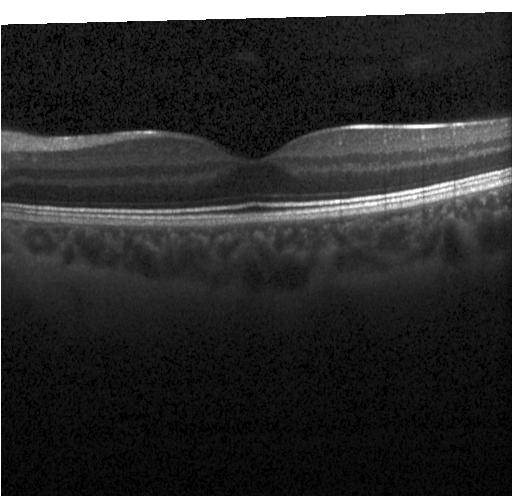
Macular scan · optical coherence tomography B-scan · spectral-domain optical coherence tomography.
Dx: neither choroidal neovascularization, diabetic macular edema, nor drusen.